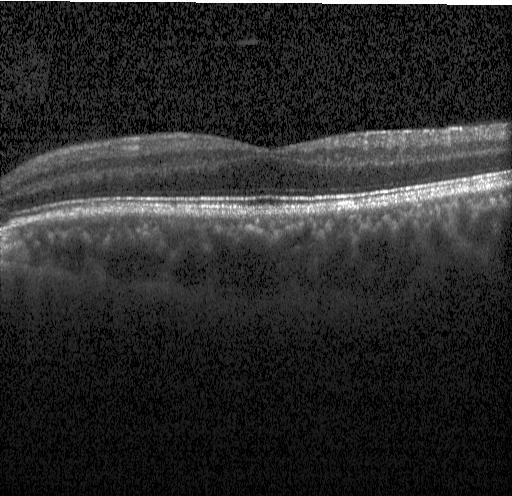
Retinal OCT cross-section showing no choroidal neovascularization, no diabetic macular edema, and no drusen.